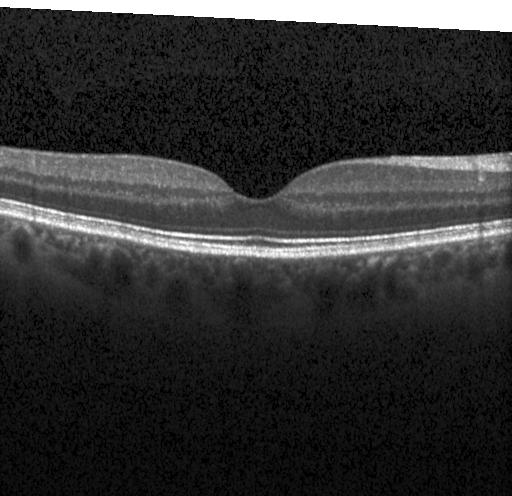

Finding: no choroidal neovascularization, no diabetic macular edema, and no drusen.